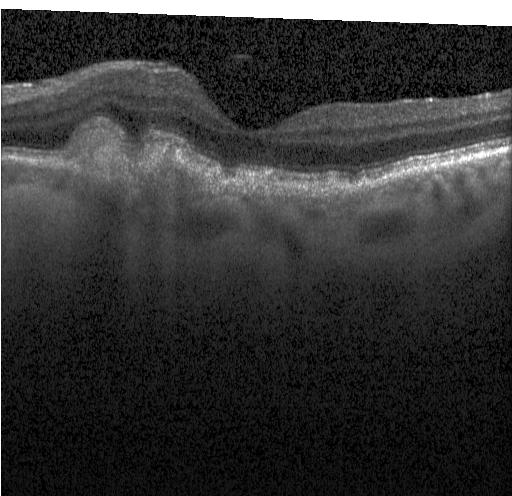

OCT B-scan
Diagnosis: choroidal neovascularization (CNV).